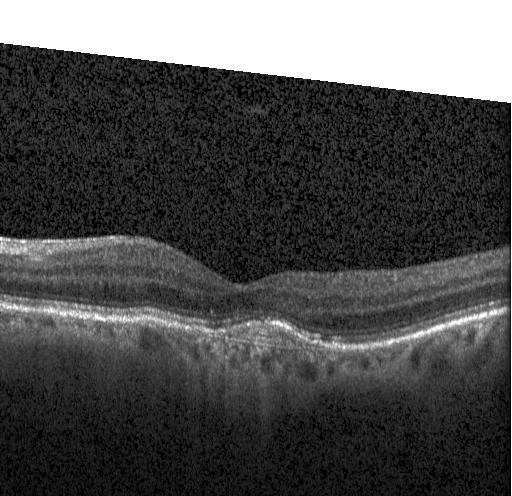
The scan shows a choroidal neovascular membrane.